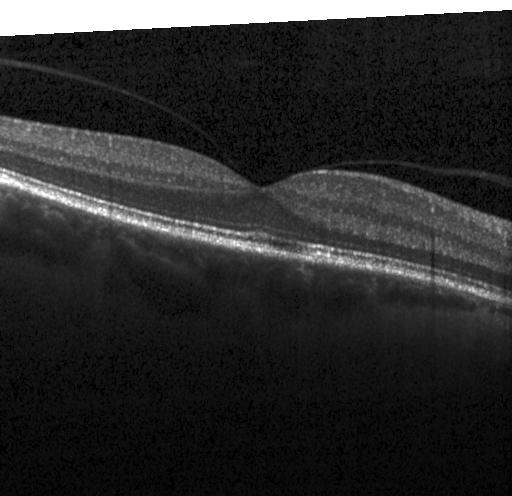

OCT B-scan — Finding: neither choroidal neovascularization, diabetic macular edema, nor drusen.